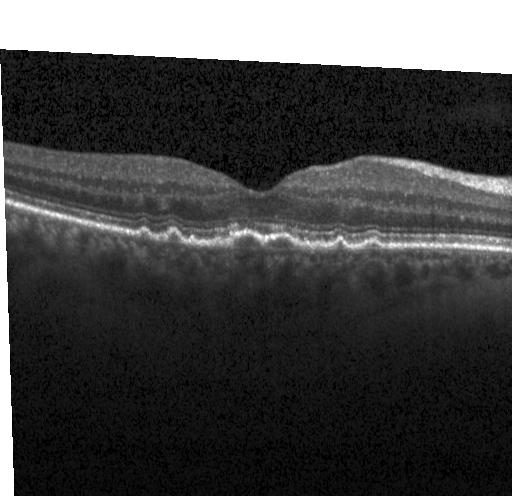
Optical coherence tomography B-scan. Impression: drusen.